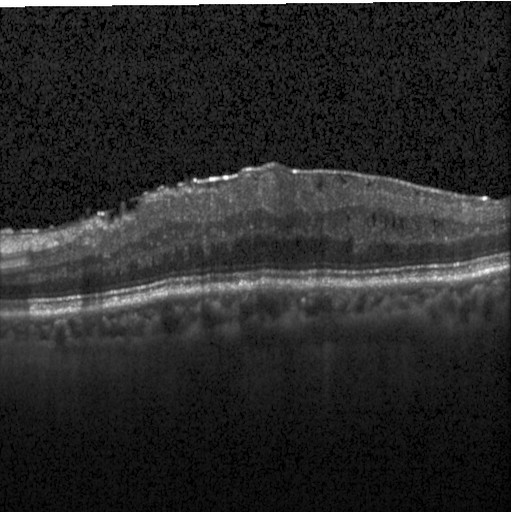
Optical coherence tomography B-scan. OCT finding: diabetic macular edema.